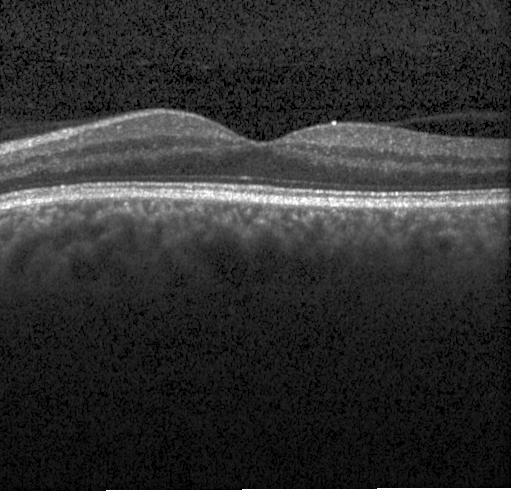 OCT line scan · macular scan — This B-scan demonstrates no evidence of choroidal neovascularization, diabetic macular edema, or drusen.